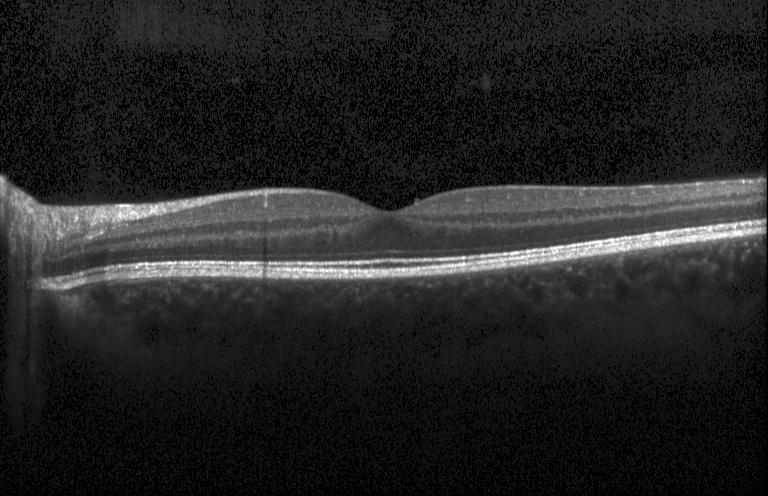 Dx: neither CNV, DME, nor drusen.